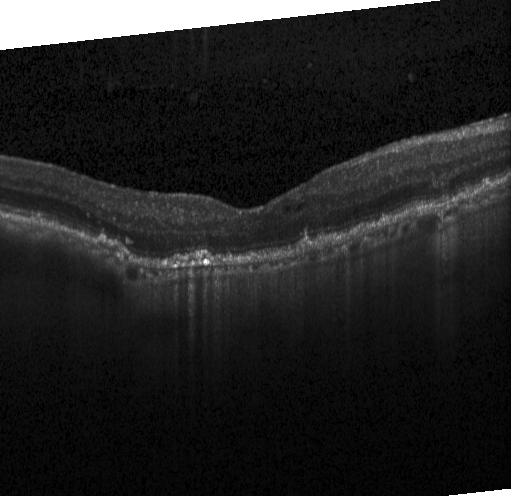
Dx: a choroidal neovascular membrane.